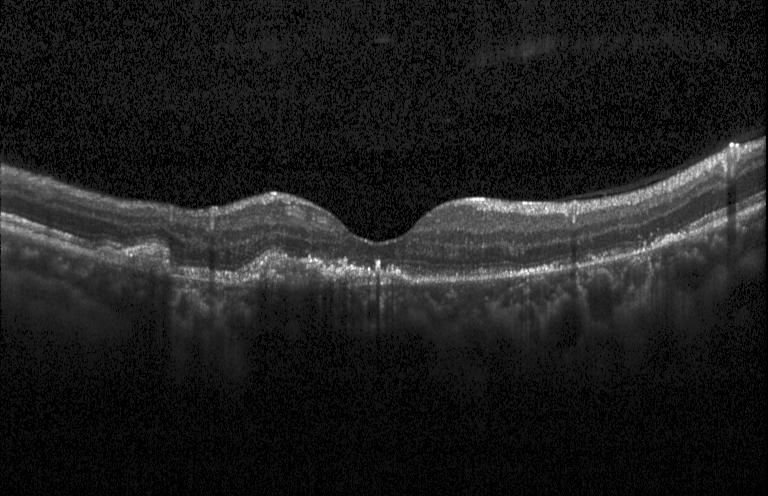

Dx: CNV.